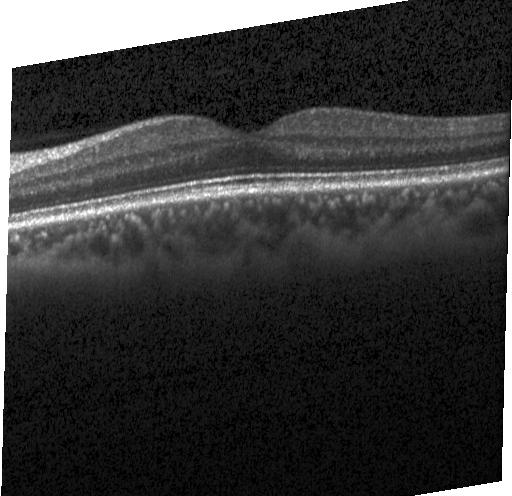 Impression: neither choroidal neovascularization, diabetic macular edema, nor drusen.